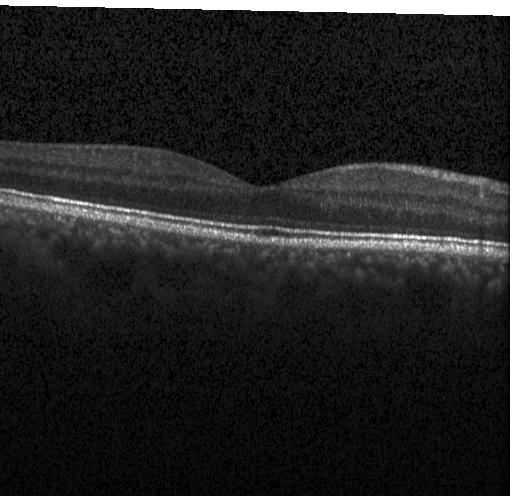
No CNV, DME, or drusen.